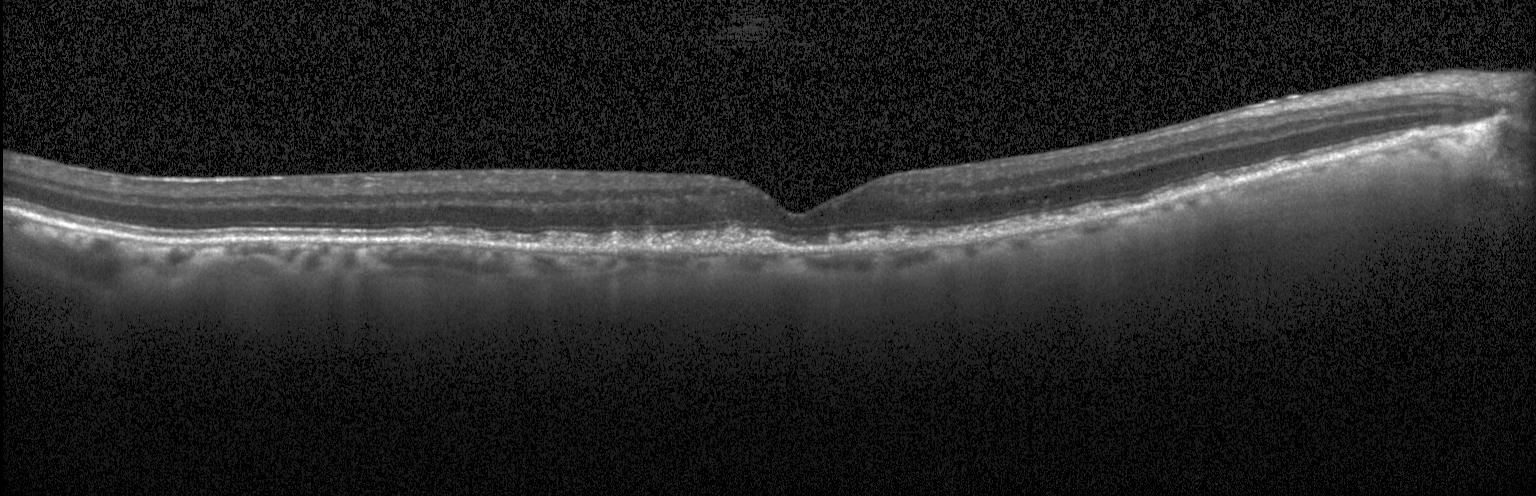 Heidelberg Spectralis. OCT line scan. SD-OCT. Drusen.